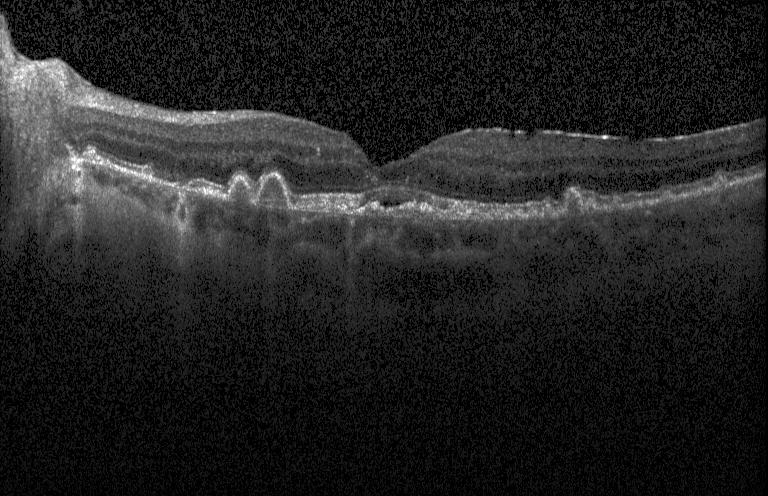
Optical coherence tomography scan; Heidelberg Spectralis OCT system
Assessment: CNV.